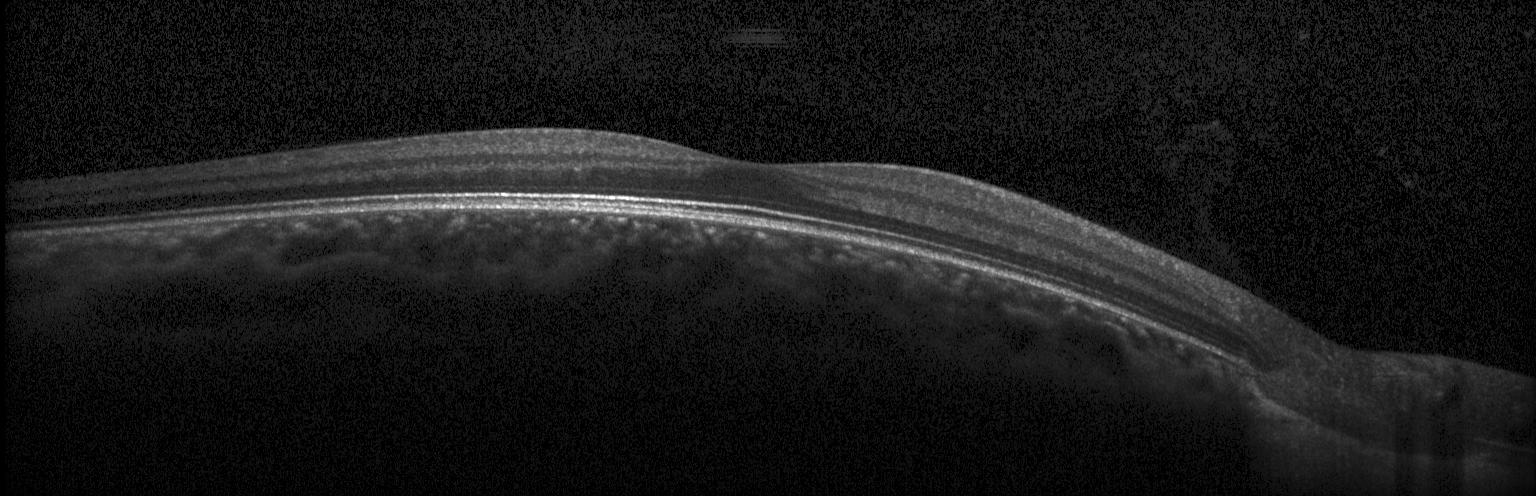
The scan shows neither choroidal neovascularization, diabetic macular edema, nor drusen.